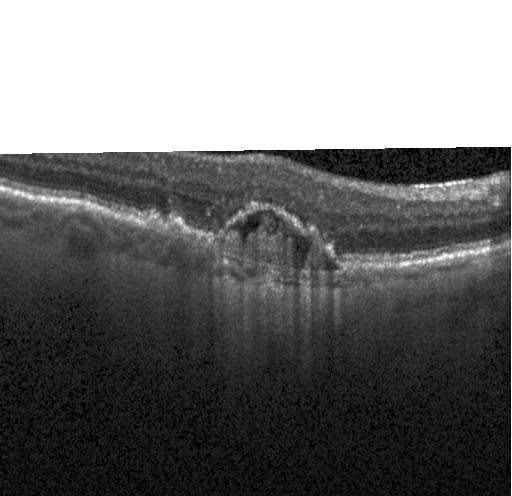
Spectral-domain optical coherence tomography · optical coherence tomography scan · through the macula · Heidelberg Spectralis.
OCT finding: a choroidal neovascular membrane.